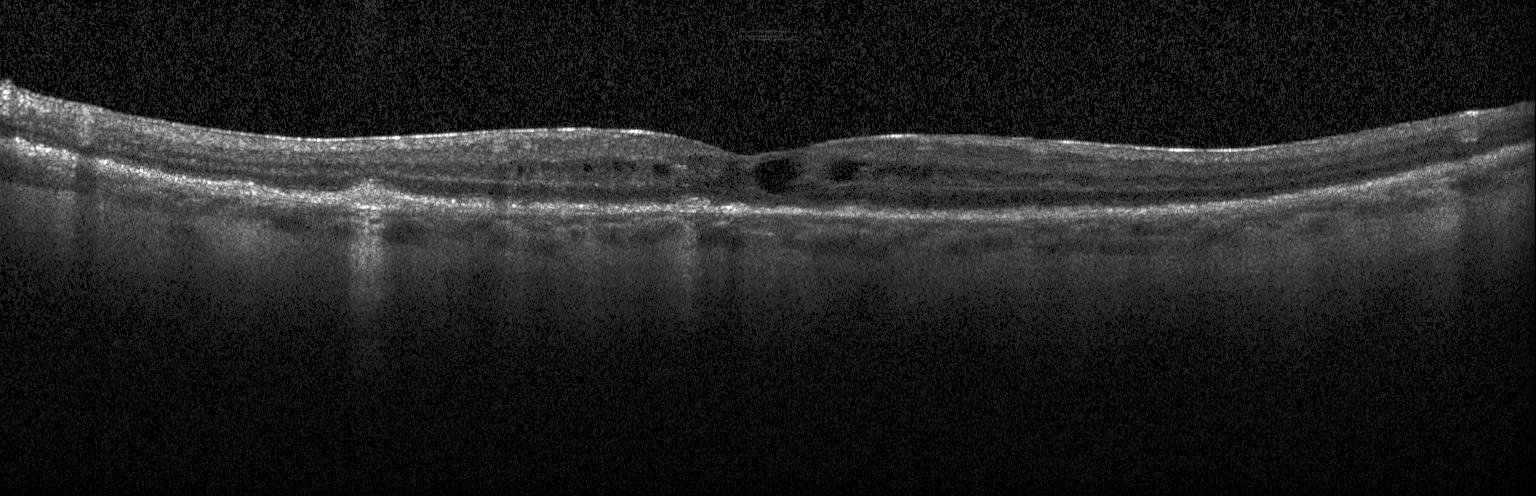

Diagnosis: choroidal neovascularization (CNV).